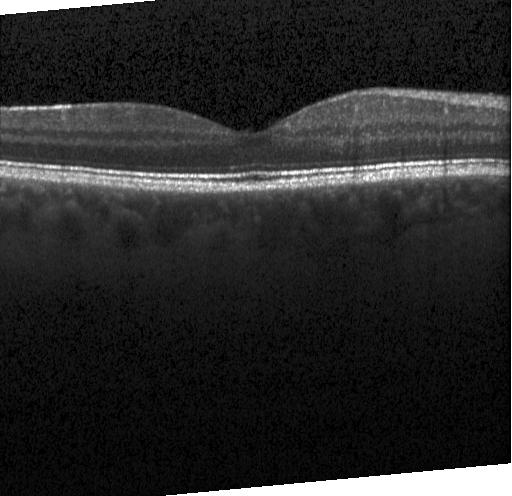
Centered on the fovea · optical coherence tomography scan · spectral-domain OCT — Diagnosis: neither choroidal neovascularization, diabetic macular edema, nor drusen.